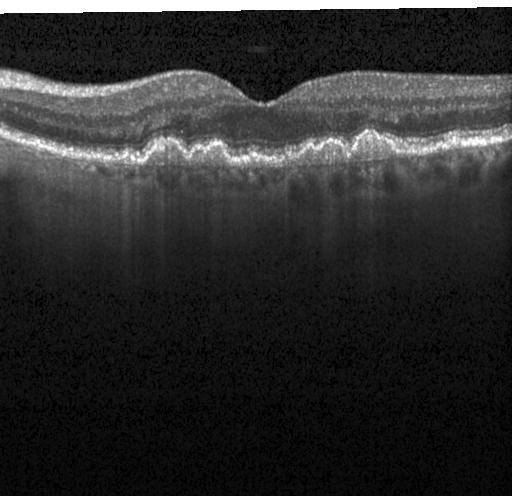
Diagnosis: multiple drusen.